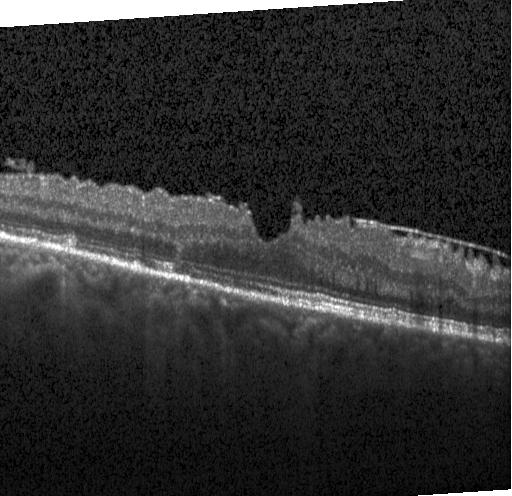

Optical coherence tomography B-scan · instrument: Heidelberg Spectralis · through the macula · SD-OCT. This B-scan demonstrates drusen.